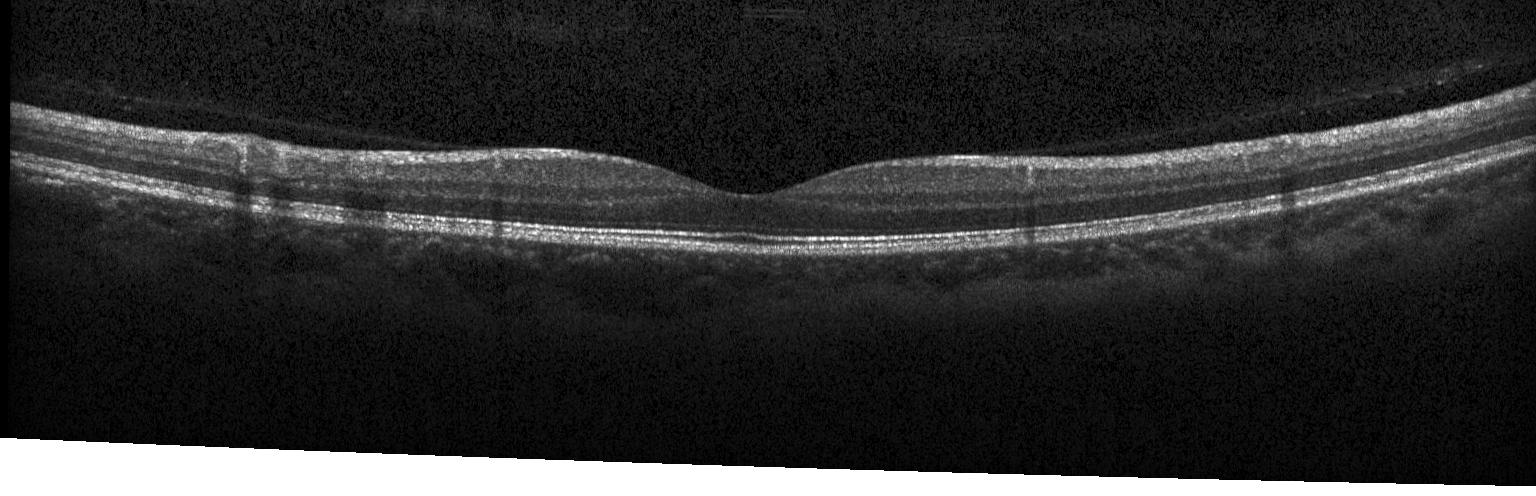

Dx: no evidence of CNV, DME, or drusen.